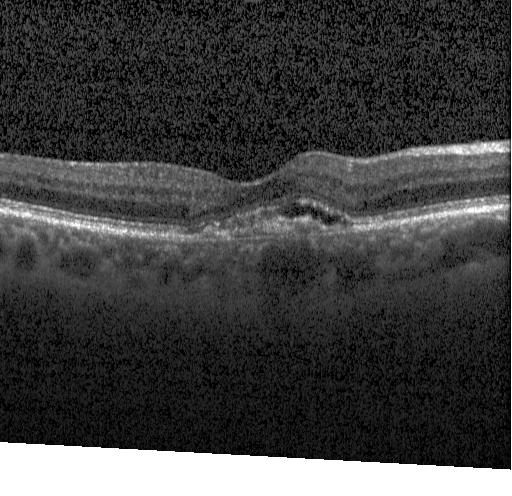

OCT finding: a choroidal neovascular membrane.